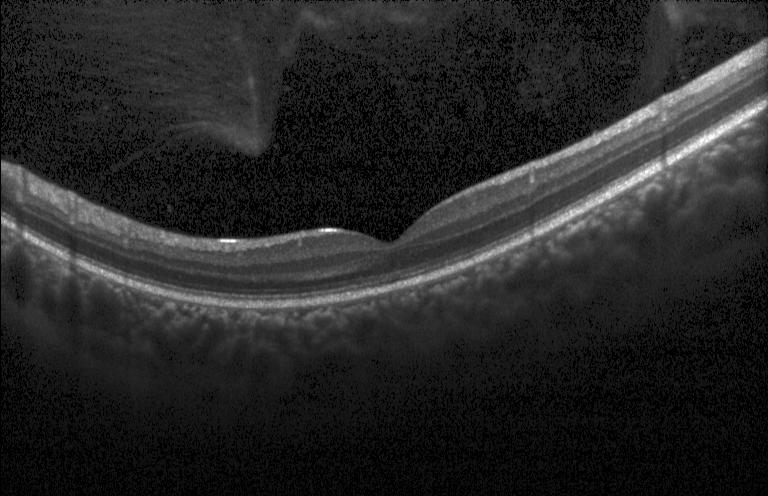 Optical coherence tomography B-scan. Diagnosis: neither choroidal neovascularization, diabetic macular edema, nor drusen.